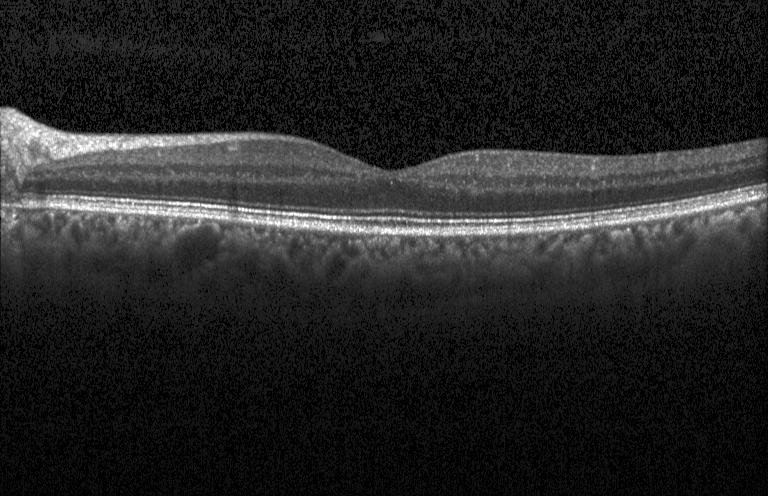
Retinal OCT cross-section
Diagnosis: no CNV, no DME, and no drusen.